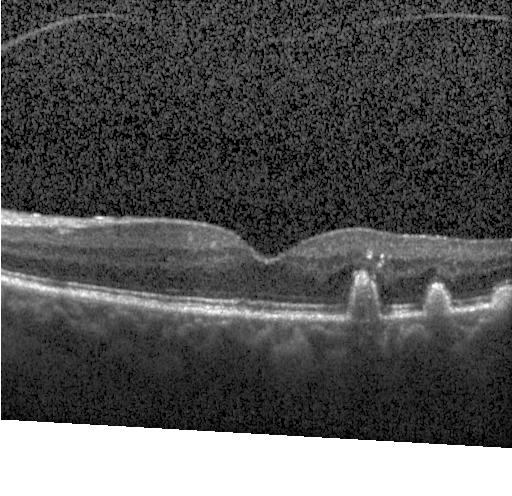
The scan shows multiple drusen.